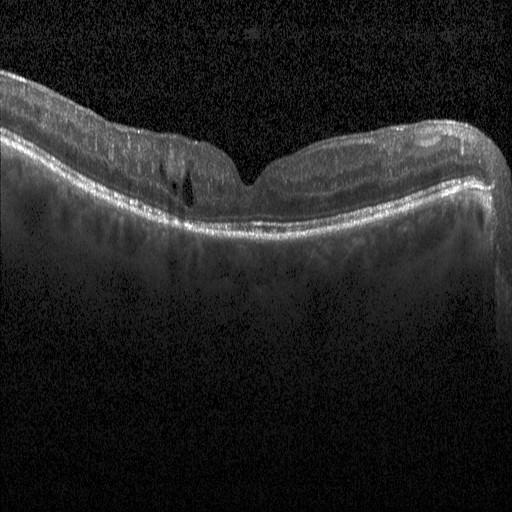

OCT line scan. Horizontal scan through the fovea. Acquired on a Heidelberg Spectralis.
Diagnosis: diabetic macular edema.